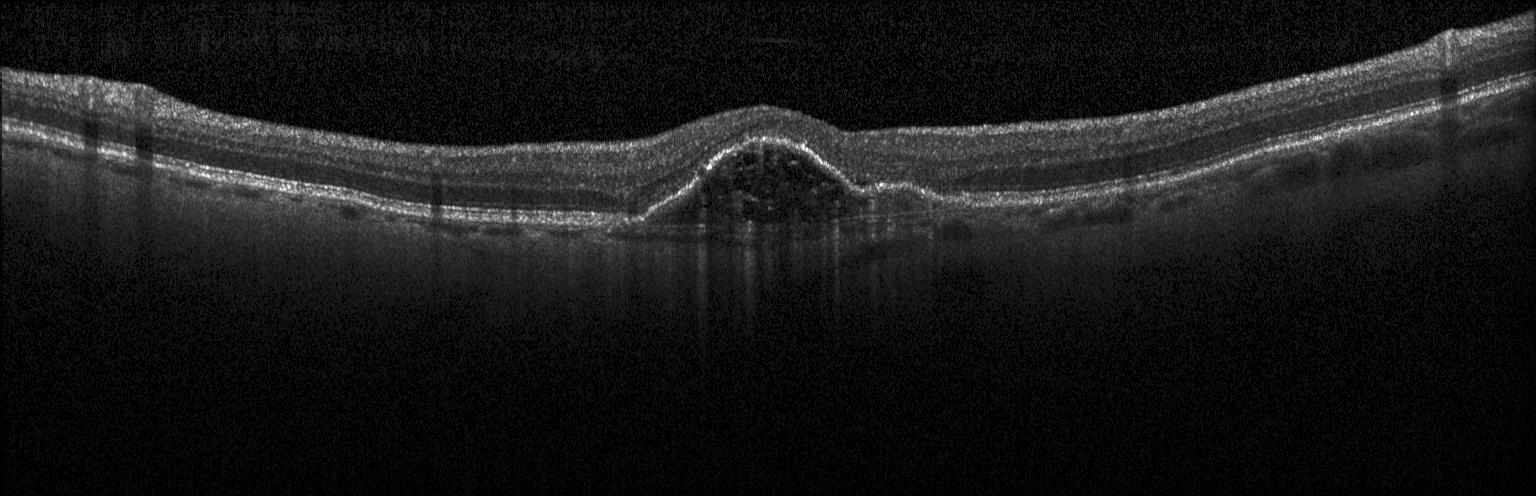
Diagnosis: a choroidal neovascular membrane.